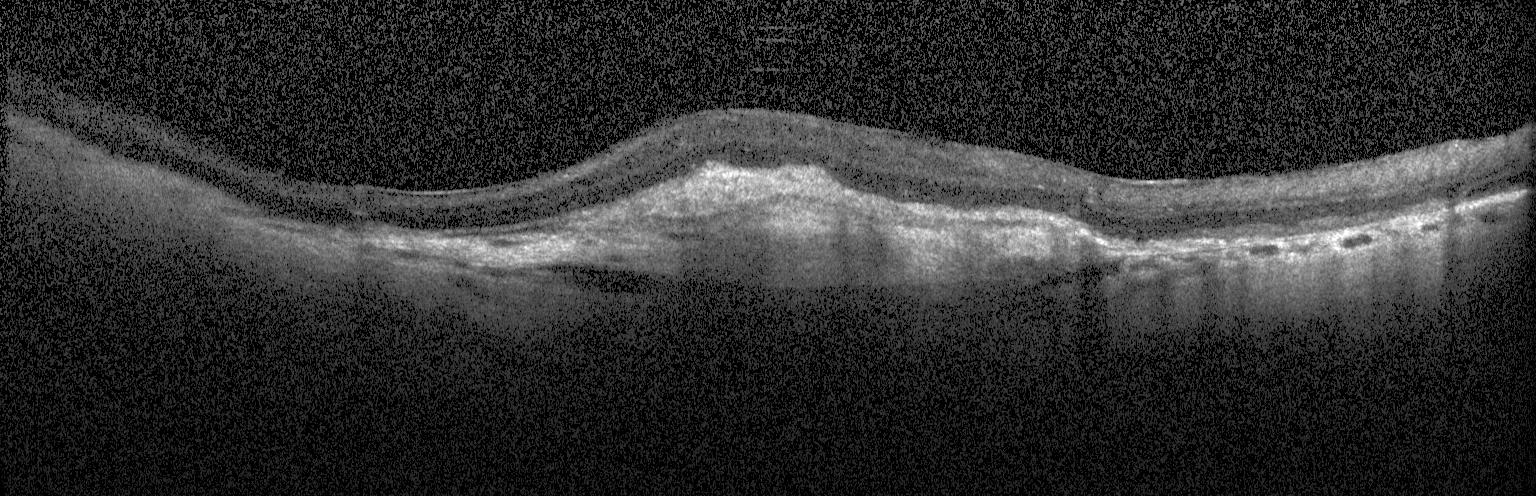

This B-scan demonstrates a choroidal neovascular membrane.